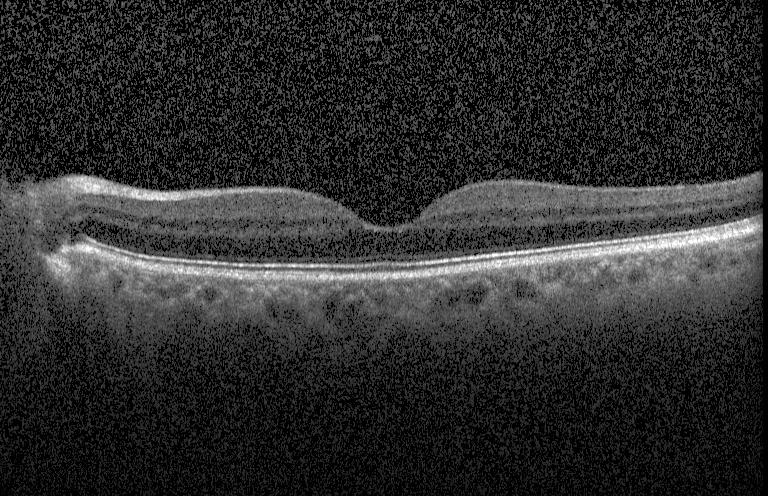
Retinal OCT B-scan — Diagnosis: no CNV, DME, or drusen.